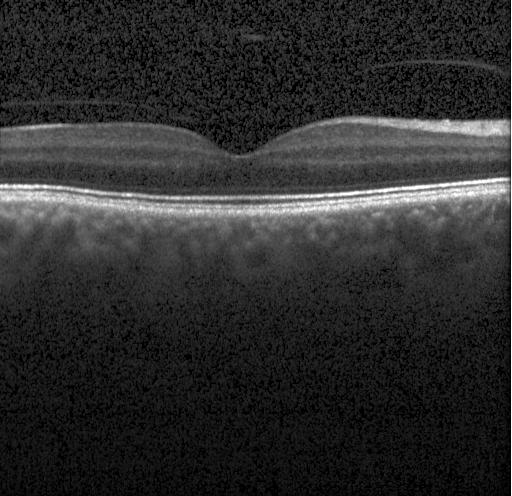 Retinal OCT cross-section · acquired on a Heidelberg Spectralis · centered on the fovea · spectral-domain OCT.
This B-scan demonstrates no choroidal neovascularization, diabetic macular edema, or drusen.